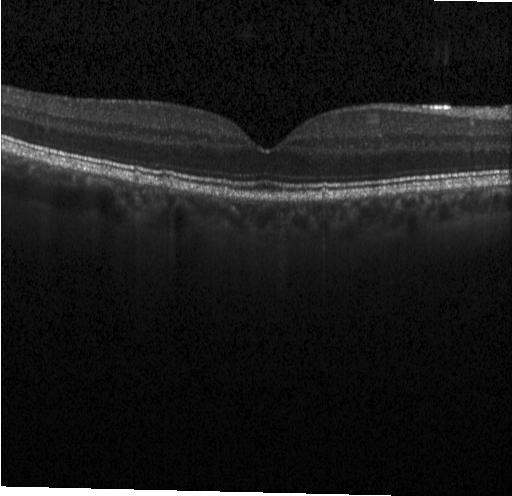
This B-scan demonstrates neither choroidal neovascularization, diabetic macular edema, nor drusen.